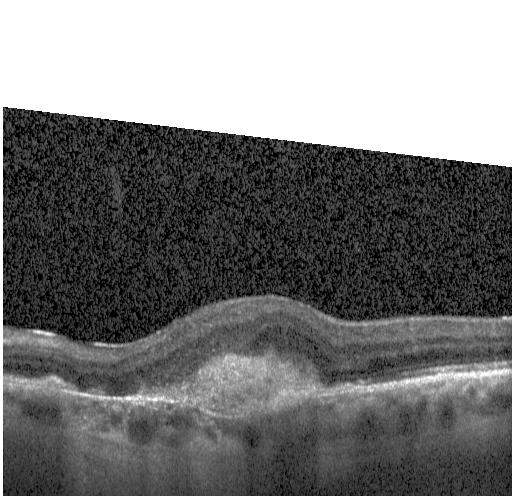
OCT B-scan. Instrument: Heidelberg Spectralis. SD-OCT. Horizontal scan through the fovea. This B-scan demonstrates CNV.